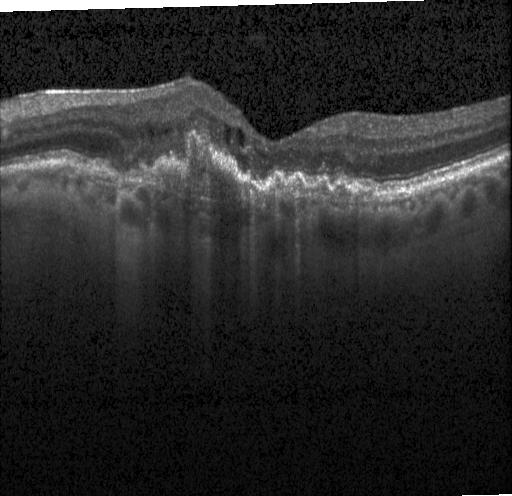

OCT line scan. Spectral-domain optical coherence tomography
OCT finding: a choroidal neovascular membrane.